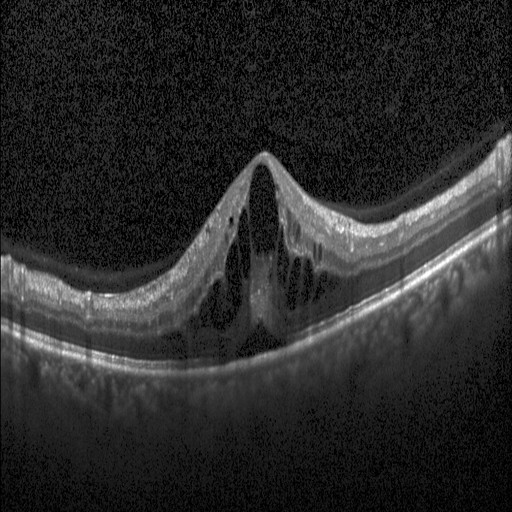

Through the macula, spectral-domain optical coherence tomography, Heidelberg Spectralis OCT system, optical coherence tomography scan.
The scan shows DME.